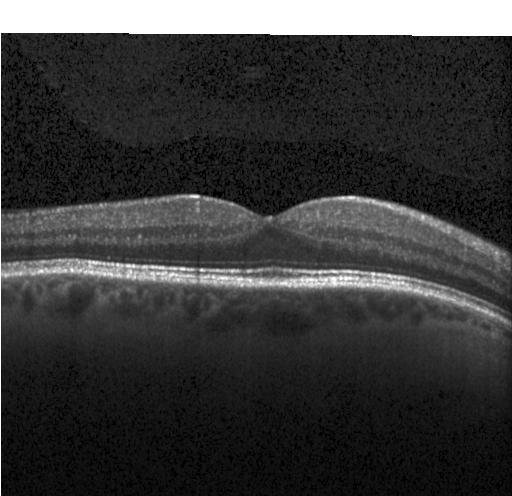

OCT B-scan showing no CNV, DME, or drusen.